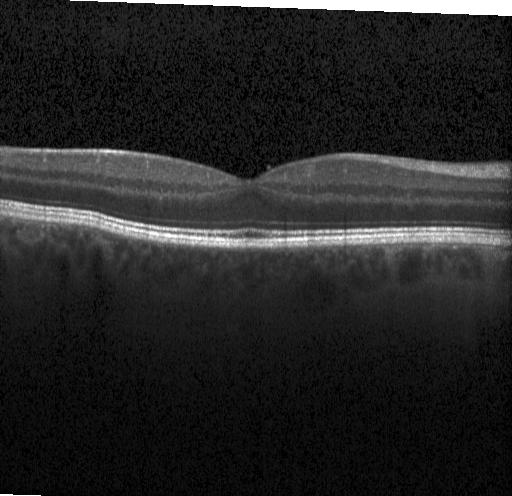

Retinal OCT cross-section. Assessment: no CNV, no DME, and no drusen.